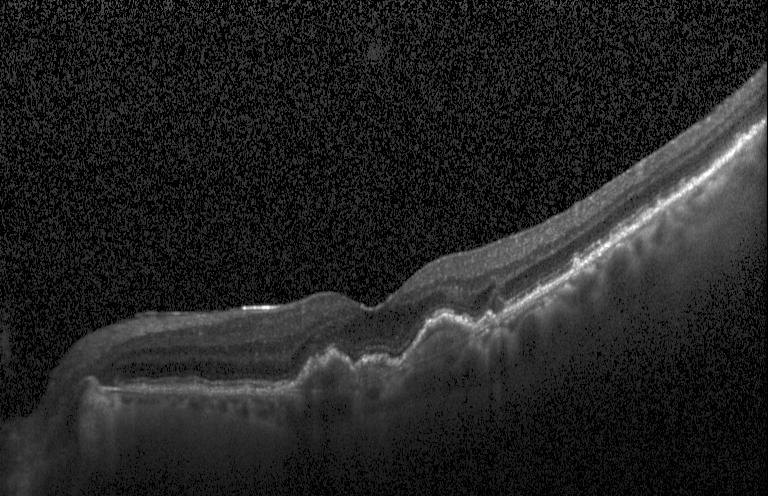
Optical coherence tomography scan. Choroidal neovascularization.